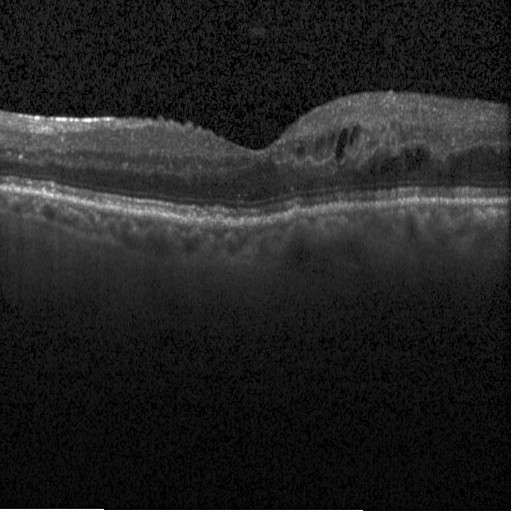 Horizontal scan through the fovea. Retinal OCT B-scan. Diagnosis: diabetic macular edema.